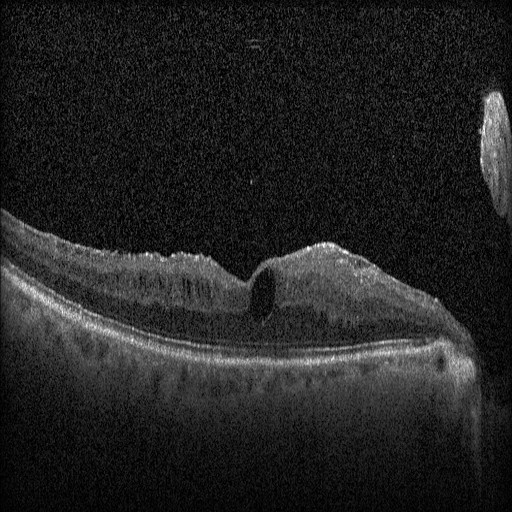
Instrument: Heidelberg Spectralis. Macular scan. Retinal OCT B-scan. This B-scan demonstrates diabetic macular edema.